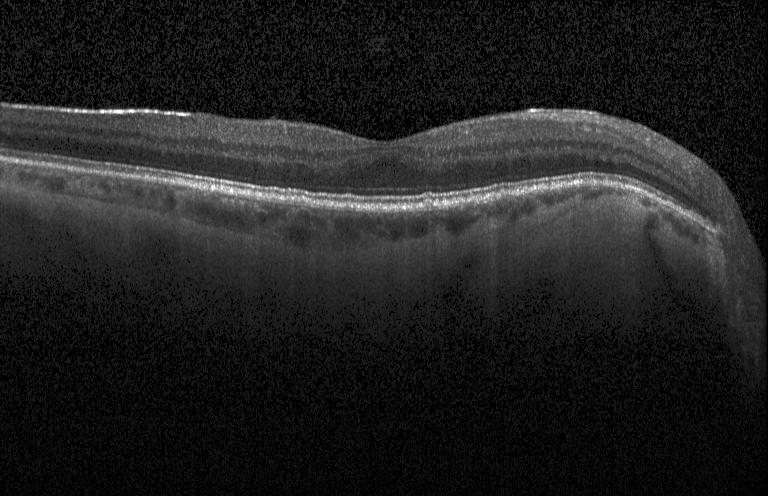

Retinal OCT B-scan. Impression: sub-RPE drusenoid deposits.